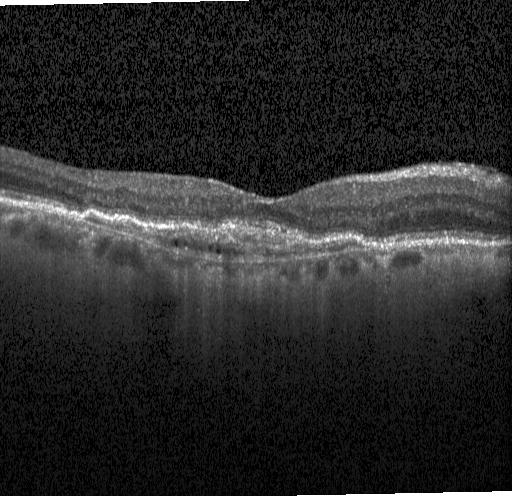 Instrument: Heidelberg Spectralis. OCT line scan. This B-scan demonstrates CNV.